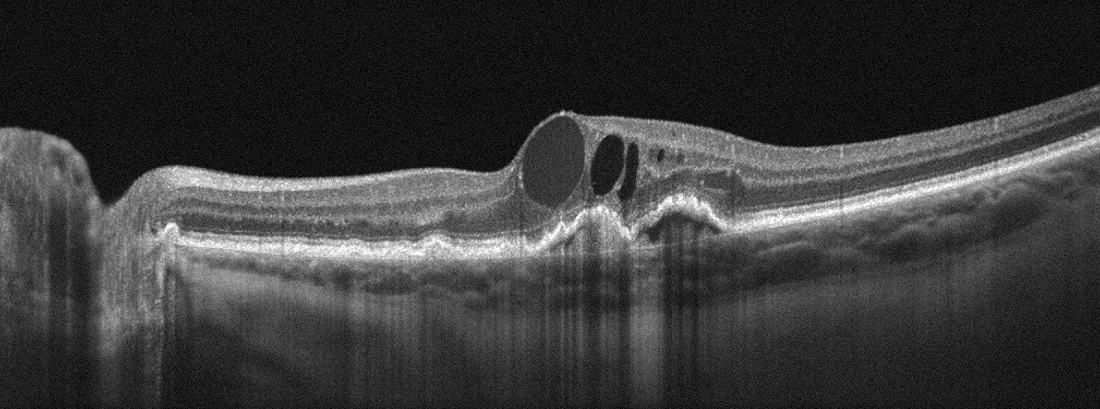

Macular scan · instrument: Optovue Avanti RTVue XR · optical coherence tomography B-scan — Assessment: age-related macular degeneration.